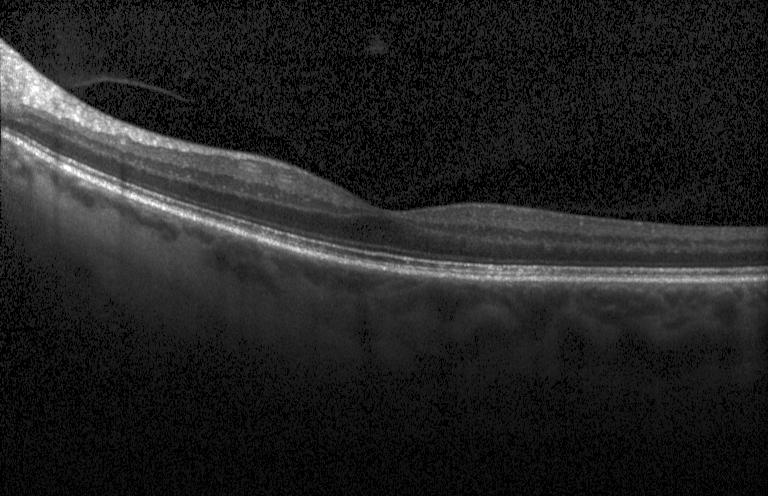
Horizontal scan through the fovea · spectral-domain optical coherence tomography · Heidelberg Spectralis · retinal OCT cross-section
Finding: no CNV, DME, or drusen.